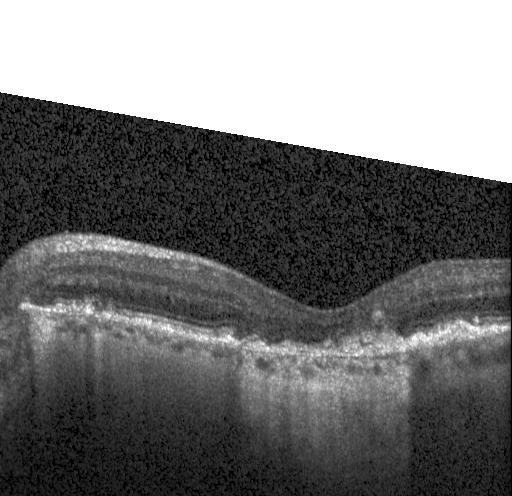 Optical coherence tomography B-scan; SD-OCT; fovea-centered — Diagnosis: CNV.